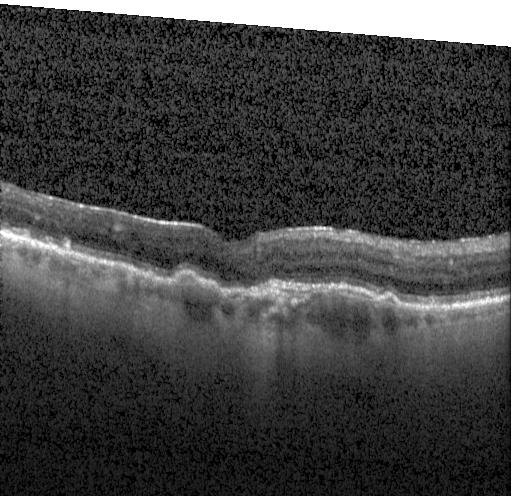 SD-OCT · optical coherence tomography scan · horizontal scan through the fovea — The scan shows a choroidal neovascular membrane.